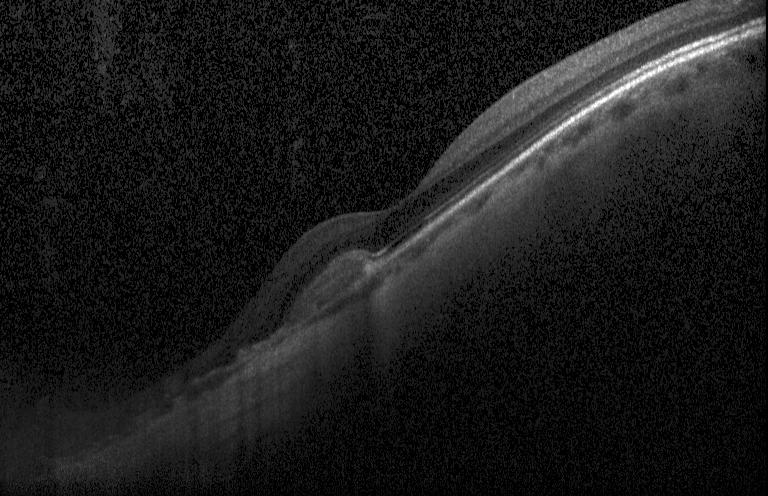 Instrument: Heidelberg Spectralis. SD-OCT. OCT line scan — Dx: a choroidal neovascular membrane.